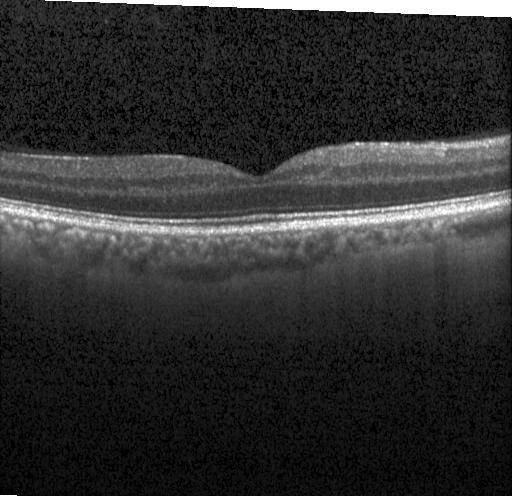
Assessment: no evidence of choroidal neovascularization, diabetic macular edema, or drusen.